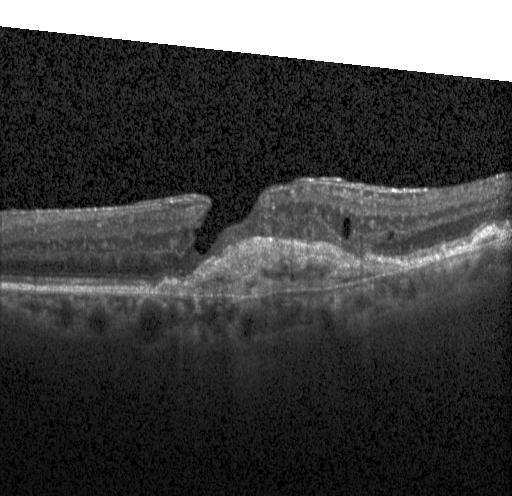

Fovea-centered, spectral-domain optical coherence tomography, optical coherence tomography B-scan. Macular OCT: choroidal neovascularization (CNV).